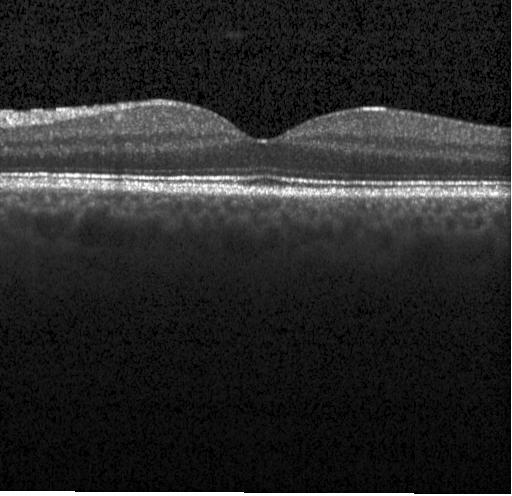

Impression: neither choroidal neovascularization, diabetic macular edema, nor drusen.